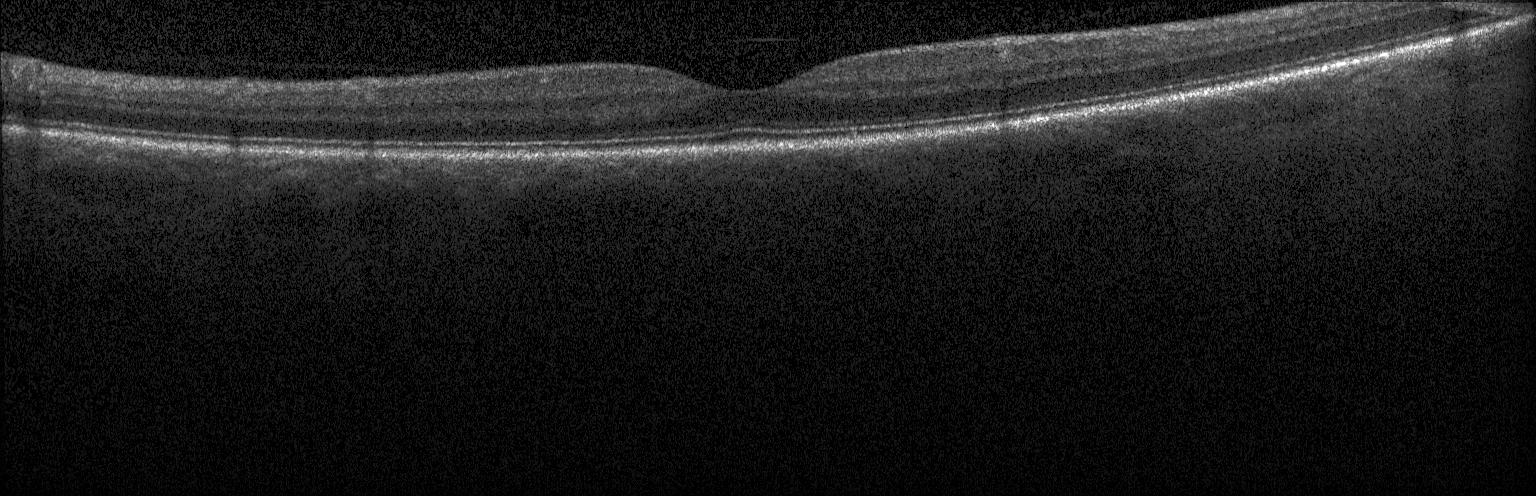 Optical coherence tomography scan
Diagnosis: neither CNV, DME, nor drusen.